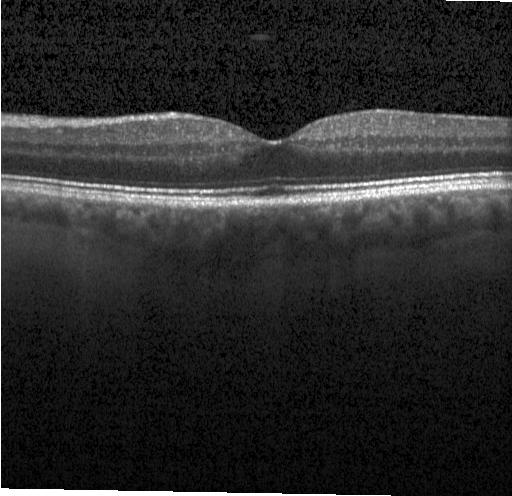 Optical coherence tomography B-scan. Diagnosis: neither choroidal neovascularization, diabetic macular edema, nor drusen.